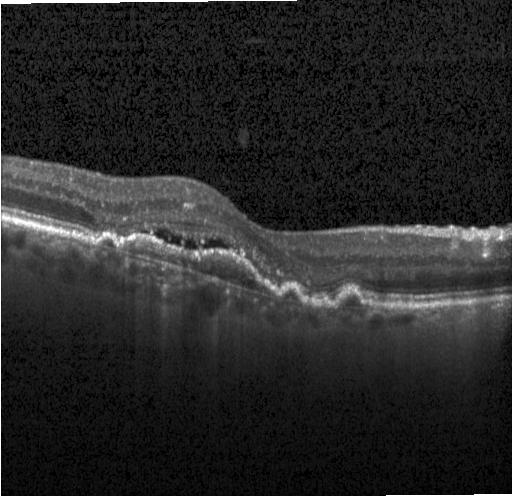
Optical coherence tomography scan.
This B-scan demonstrates CNV.